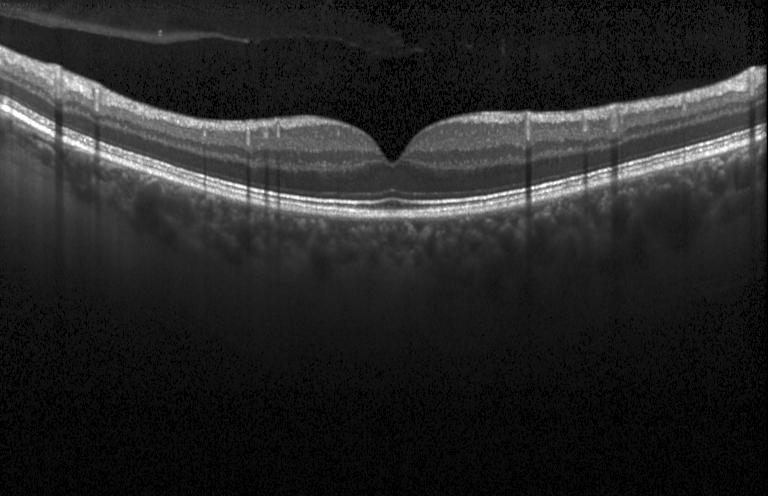
OCT B-scan — No choroidal neovascularization, no diabetic macular edema, and no drusen.